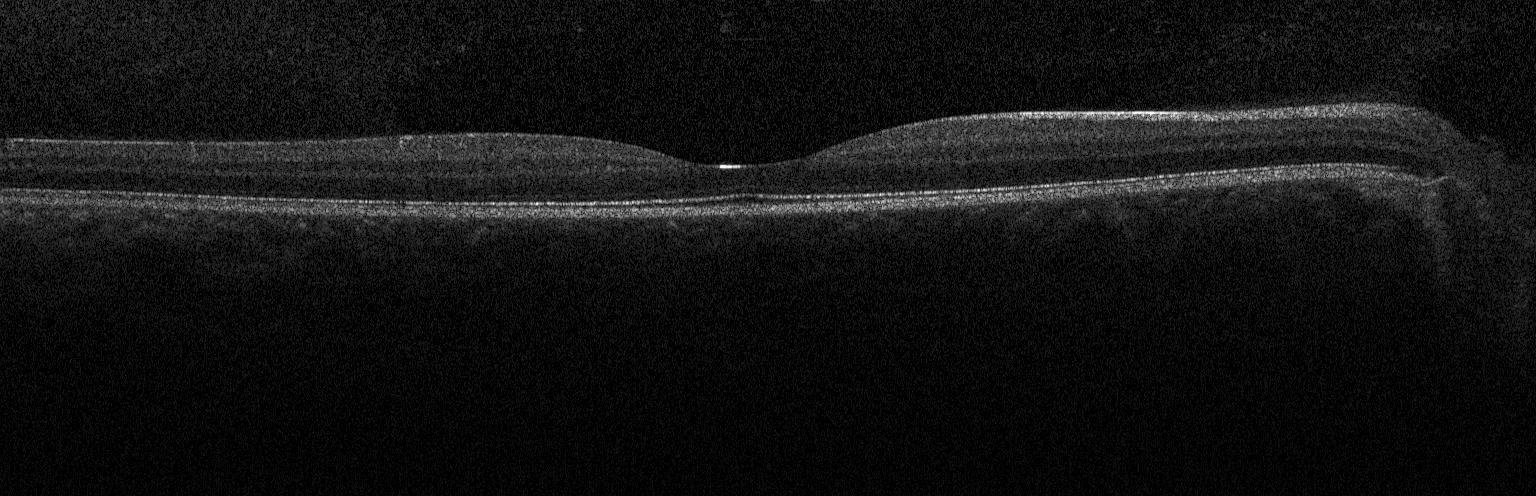
Diagnosis: no choroidal neovascularization, no diabetic macular edema, and no drusen.